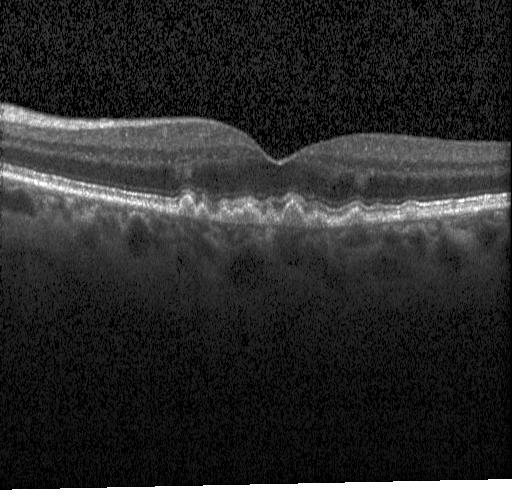

Spectral-domain optical coherence tomography. Optical coherence tomography scan.
Finding: sub-RPE drusenoid deposits.